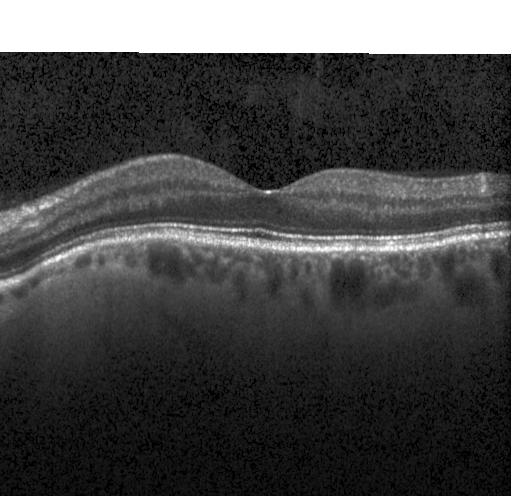 Instrument: Heidelberg Spectralis · optical coherence tomography scan · SD-OCT · centered on the fovea.
Finding: no evidence of choroidal neovascularization, diabetic macular edema, or drusen.